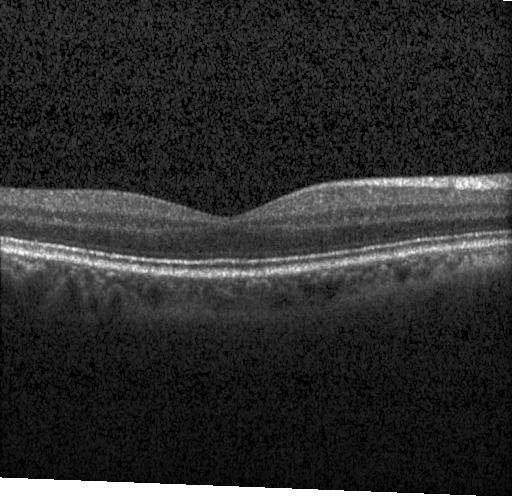

Horizontal scan through the fovea. OCT line scan. Acquired on a Heidelberg Spectralis.
Finding: neither choroidal neovascularization, diabetic macular edema, nor drusen.